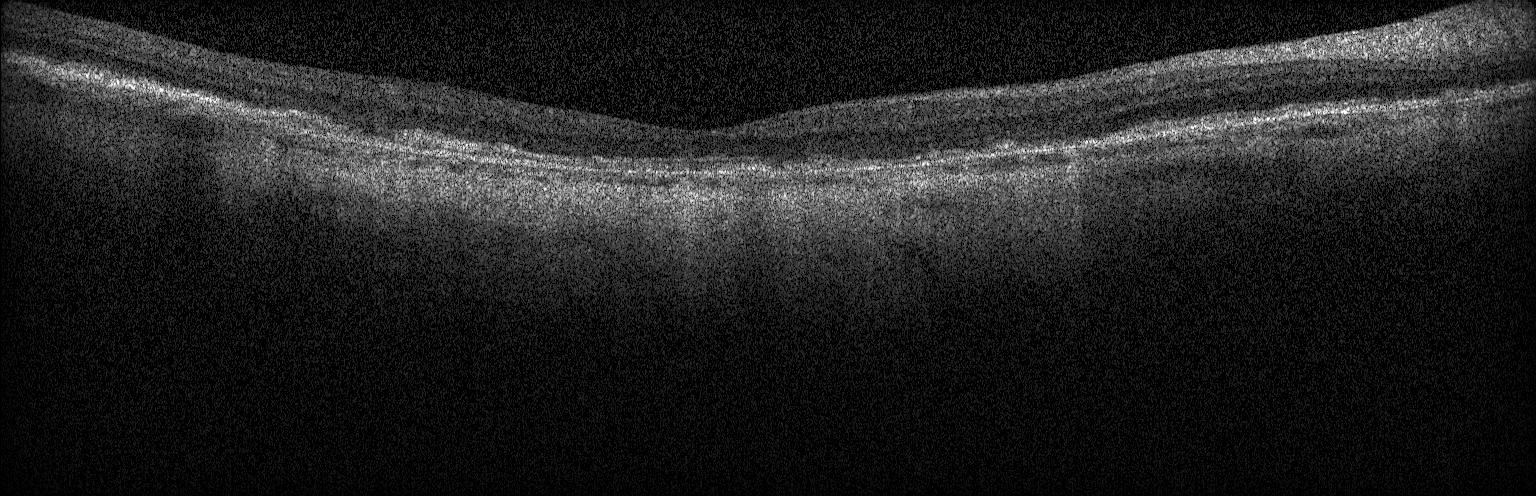
Optical coherence tomography scan, SD-OCT
OCT finding: a choroidal neovascular membrane.